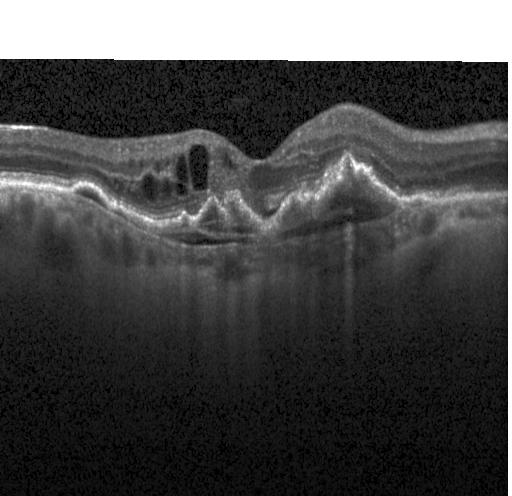 Diagnosis: a choroidal neovascular membrane.